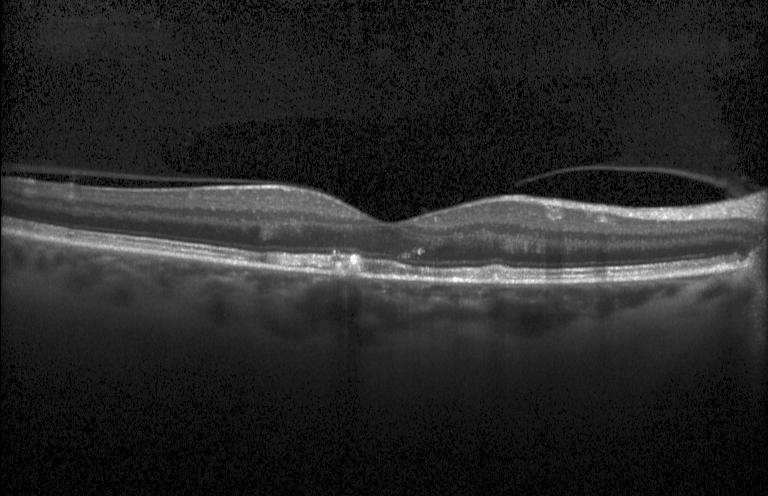
The scan shows multiple drusen.